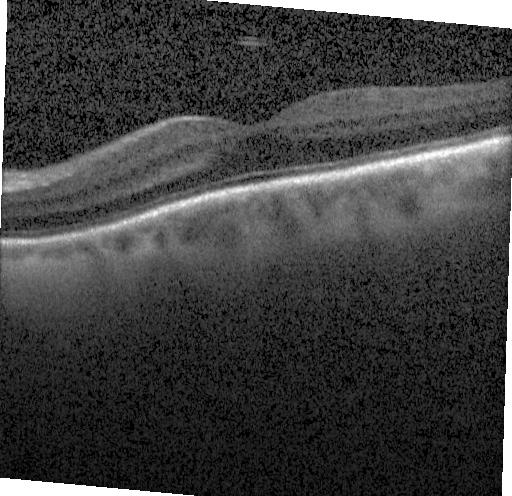

Horizontal scan through the fovea · Heidelberg Spectralis · retinal OCT B-scan — Neither choroidal neovascularization, diabetic macular edema, nor drusen.